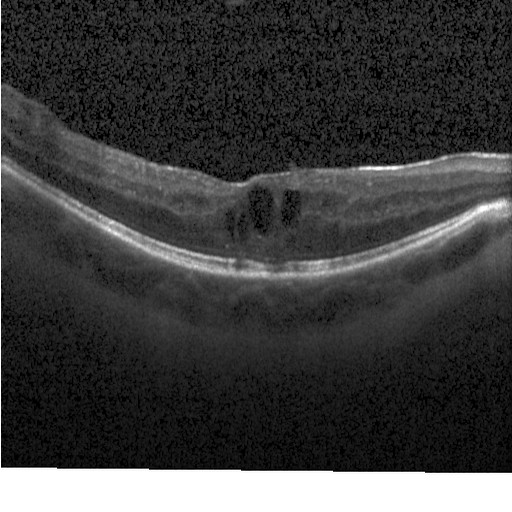 Spectral-domain OCT; retinal OCT cross-section; acquired on a Heidelberg Spectralis — Diagnosis: DME.